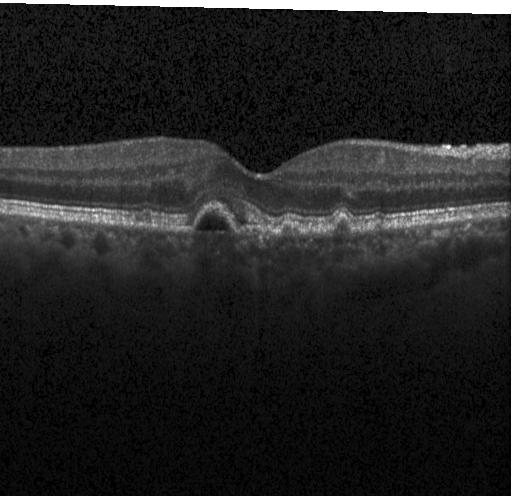
Finding: a choroidal neovascular membrane.